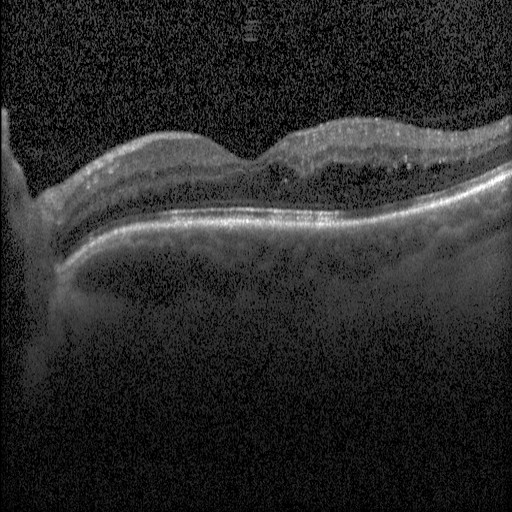
Retinal OCT B-scan
The scan shows diabetic macular edema (DME).